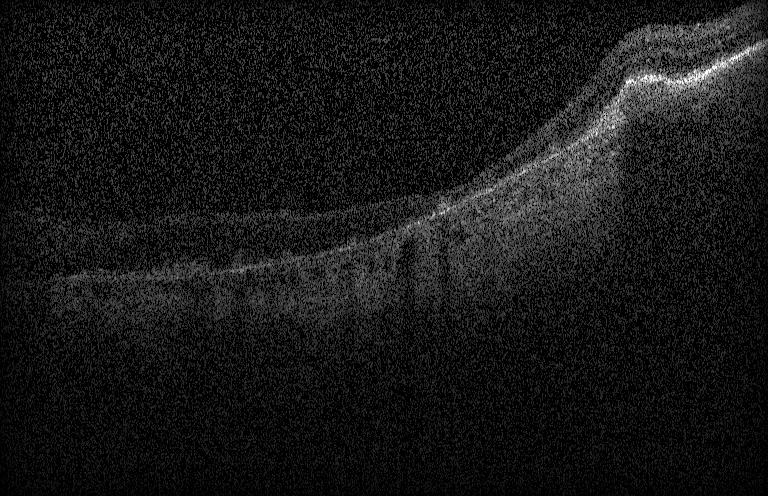
Retinal OCT cross-section showing choroidal neovascularization (CNV).